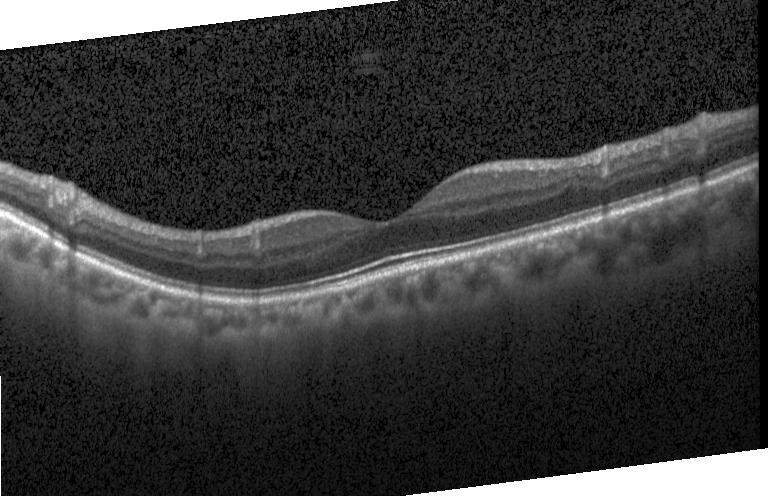 Centered on the fovea; OCT line scan; spectral-domain optical coherence tomography.
No choroidal neovascularization, diabetic macular edema, or drusen.